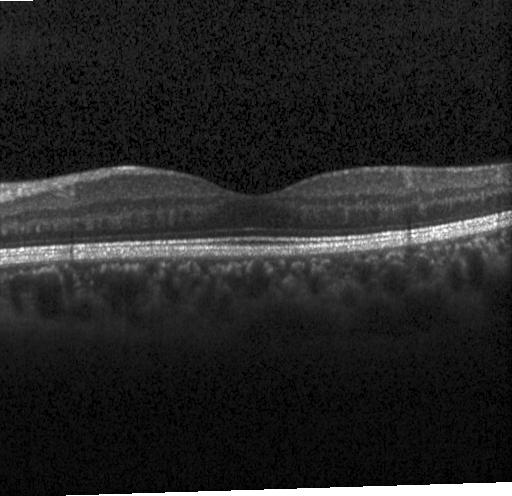 Macular scan; Heidelberg Spectralis OCT system; optical coherence tomography B-scan; SD-OCT — Diagnosis: no choroidal neovascularization, no diabetic macular edema, and no drusen.